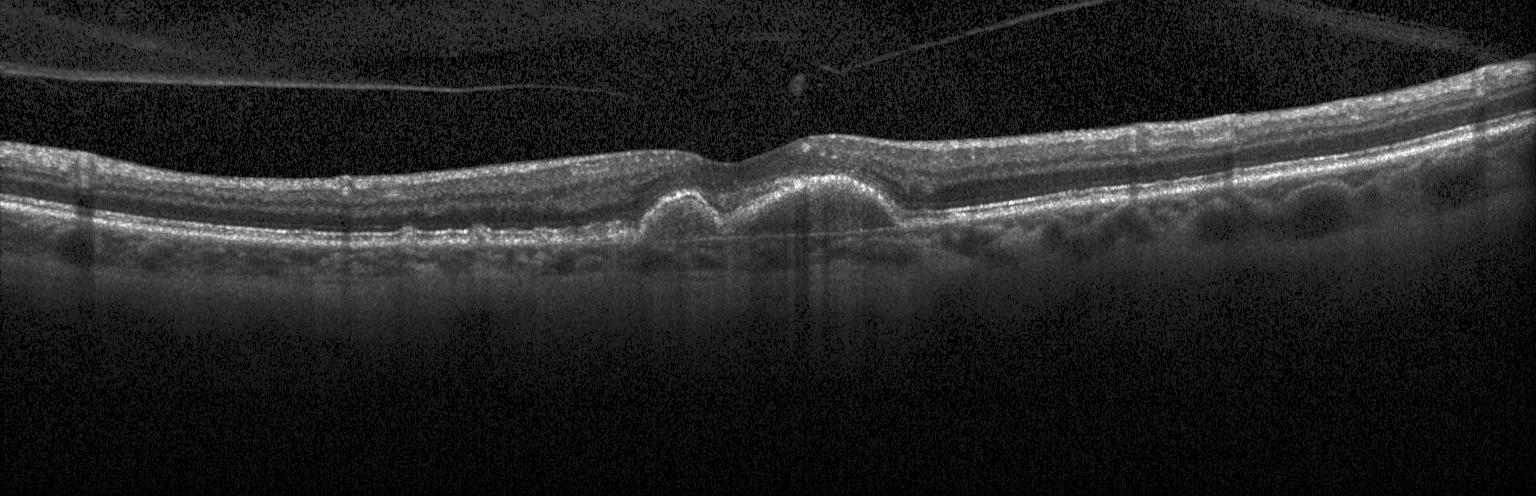
OCT B-scan. Heidelberg Spectralis OCT system
Diagnosis: a choroidal neovascular membrane.